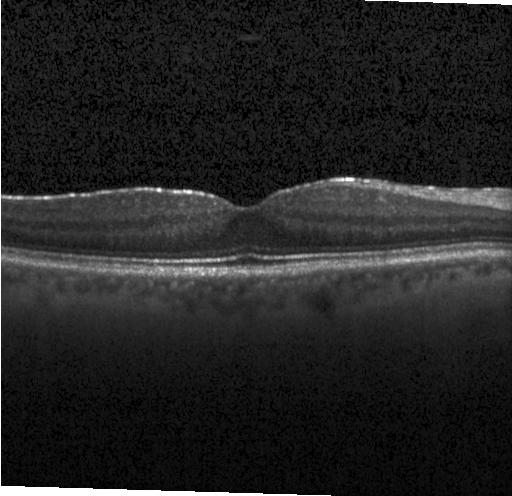 Optical coherence tomography B-scan. Impression: no evidence of choroidal neovascularization, diabetic macular edema, or drusen.